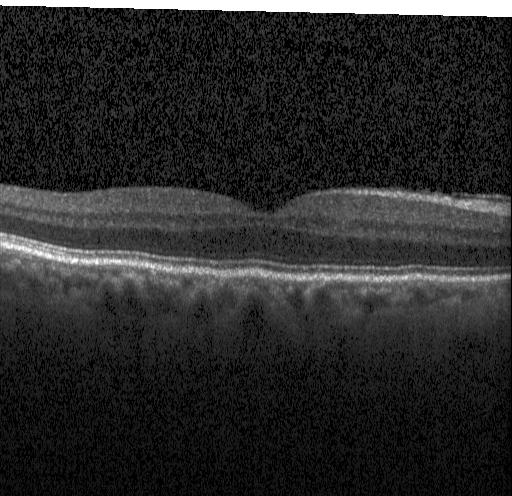

OCT line scan; centered on the fovea; SD-OCT; instrument: Heidelberg Spectralis
This B-scan demonstrates no CNV, no DME, and no drusen.